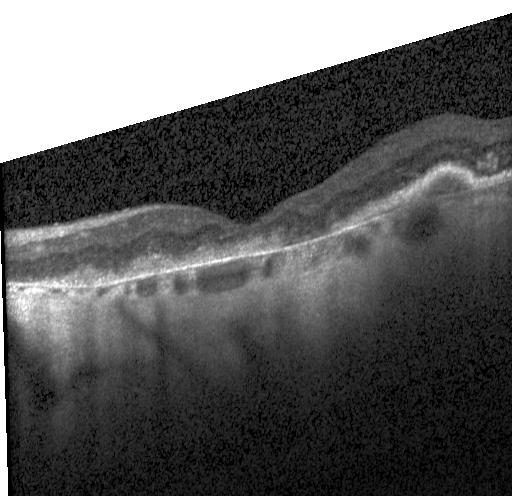 Finding: choroidal neovascularization.